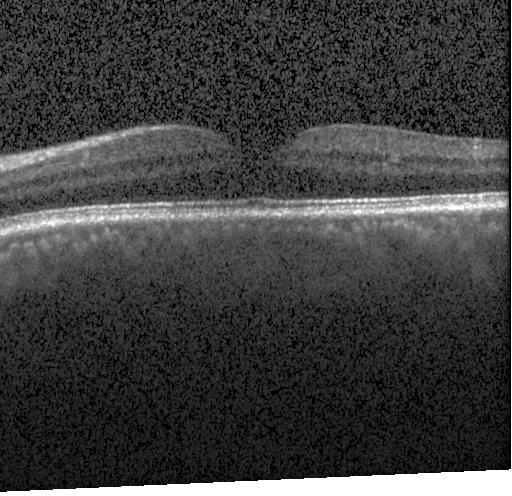
Spectral-domain OCT · optical coherence tomography scan — Finding: no choroidal neovascularization, no diabetic macular edema, and no drusen.